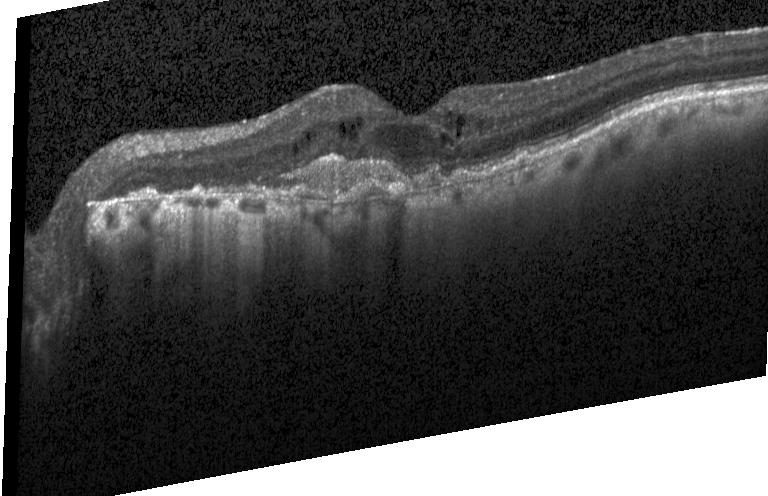
Spectral-domain OCT B-scan: a choroidal neovascular membrane.